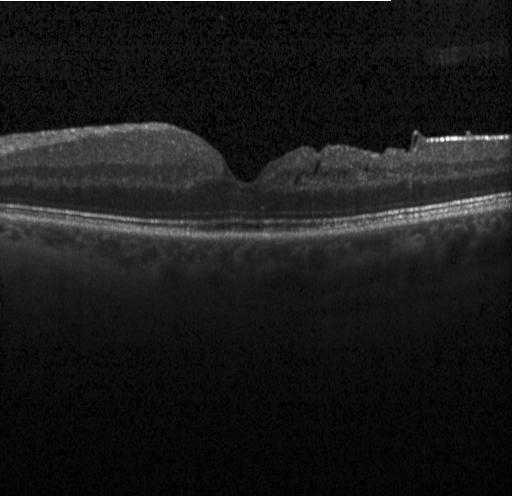
OCT B-scan showing diabetic macular edema (DME).